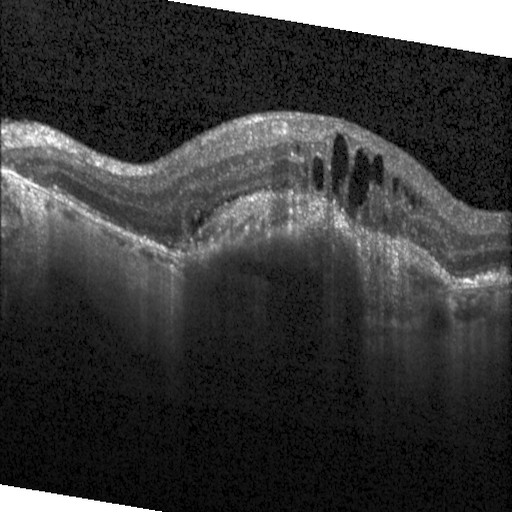
Retinal OCT cross-section showing diabetic macular edema (DME).